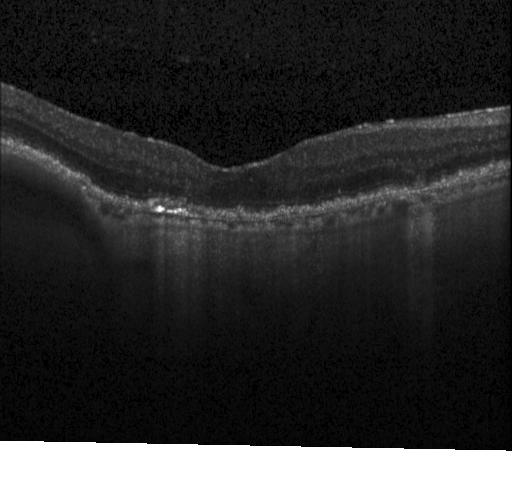

OCT B-scan — Finding: CNV.